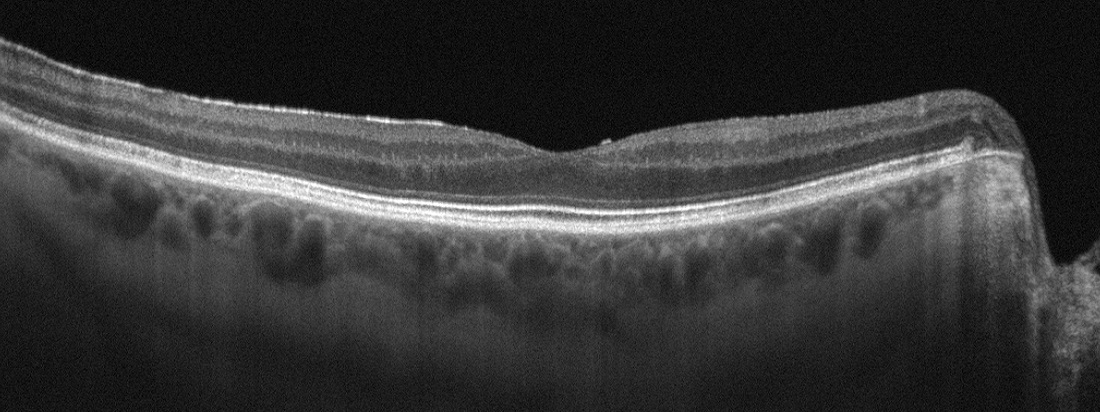
OCT line scan. Fovea-centered. Acquired on an Optovue Avanti RTVue XR
Impression: epiretinal membrane (ERM).